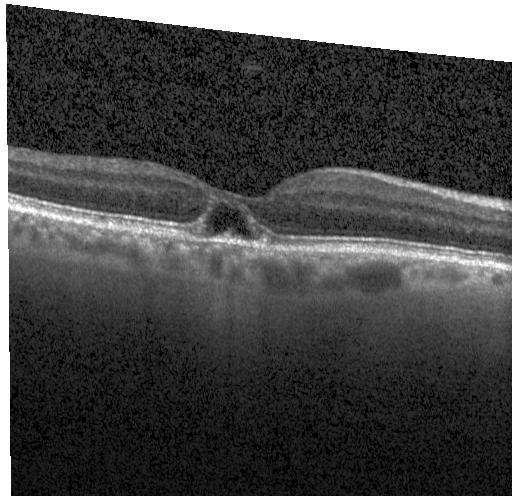

OCT finding: choroidal neovascularization (CNV).